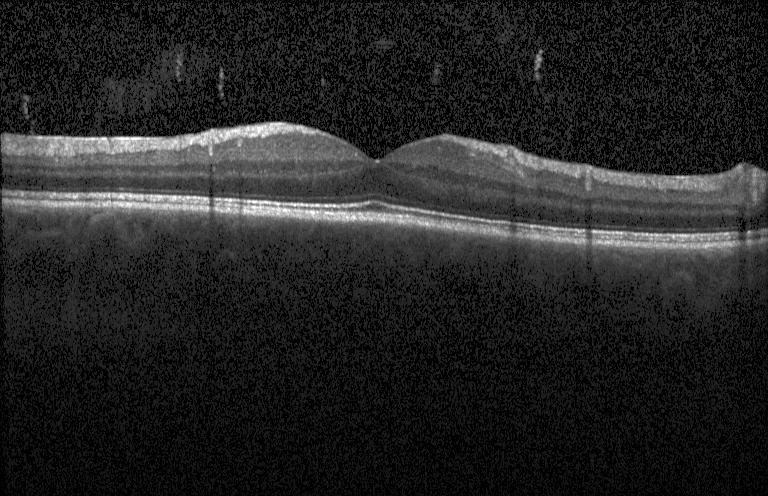

SD-OCT, optical coherence tomography B-scan.
Impression: neither choroidal neovascularization, diabetic macular edema, nor drusen.